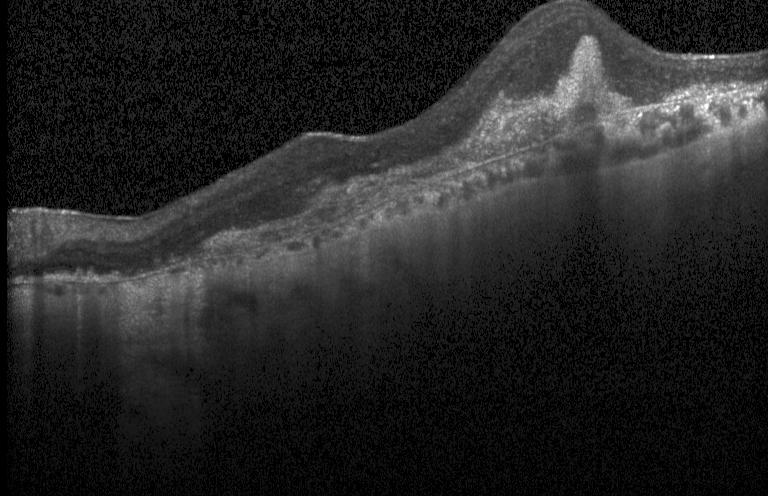

OCT line scan, instrument: Heidelberg Spectralis, spectral-domain optical coherence tomography, fovea-centered — OCT finding: a choroidal neovascular membrane.